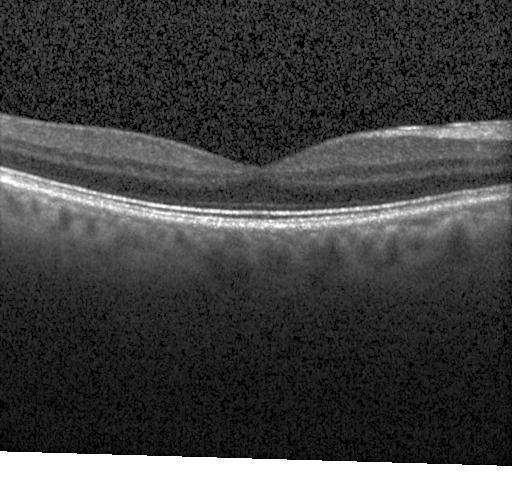

Centered on the fovea. Optical coherence tomography B-scan. Heidelberg Spectralis OCT system. Spectral-domain optical coherence tomography
Finding: no evidence of choroidal neovascularization, diabetic macular edema, or drusen.